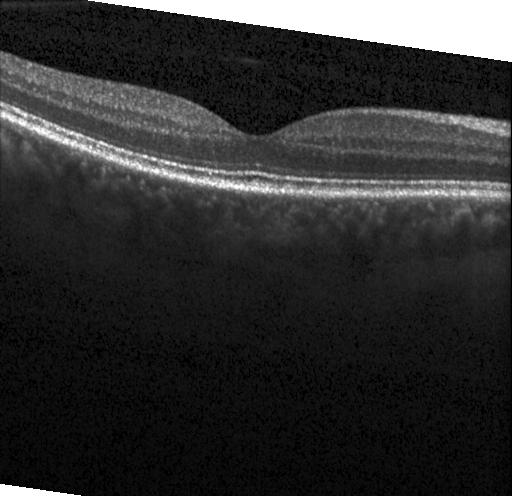 Retinal OCT B-scan — Finding: neither choroidal neovascularization, diabetic macular edema, nor drusen.